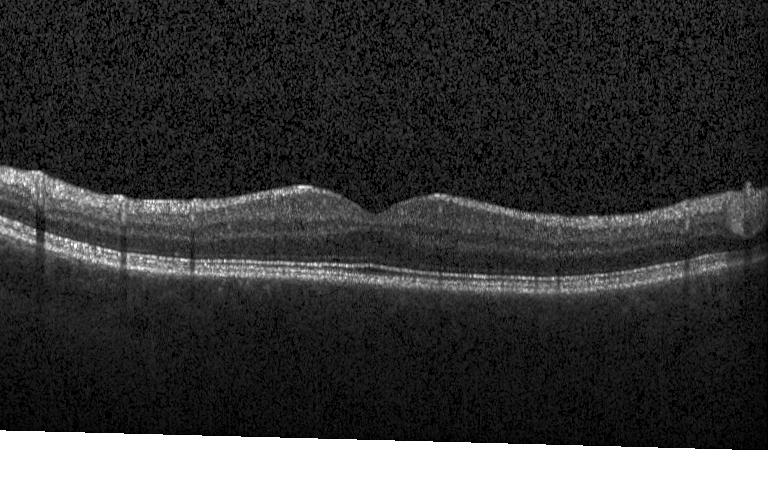 Impression: neither choroidal neovascularization, diabetic macular edema, nor drusen.